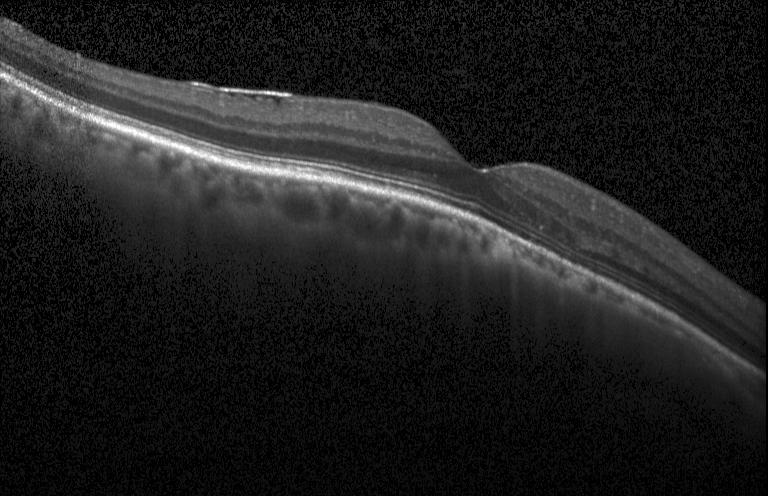
Impression: neither choroidal neovascularization, diabetic macular edema, nor drusen.